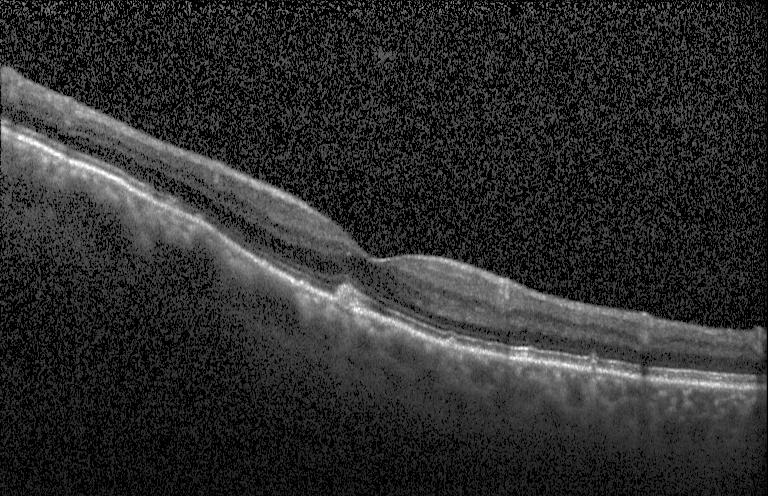 Optical coherence tomography B-scan; Heidelberg Spectralis; spectral-domain optical coherence tomography; horizontal scan through the fovea — Macular OCT: sub-RPE drusenoid deposits.